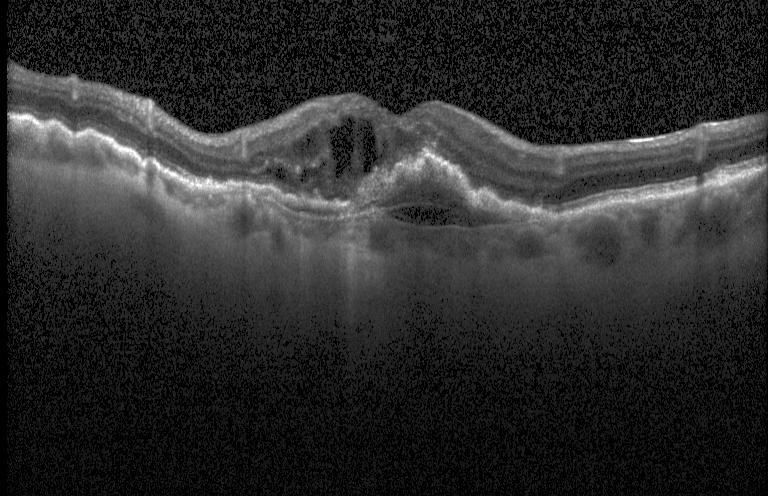
Macular scan. Retinal OCT B-scan. Instrument: Heidelberg Spectralis. Spectral-domain optical coherence tomography
Macular OCT: a choroidal neovascular membrane.